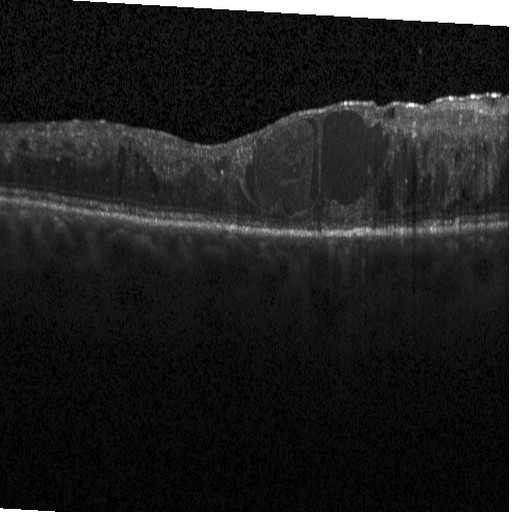 Dx: diabetic macular edema.